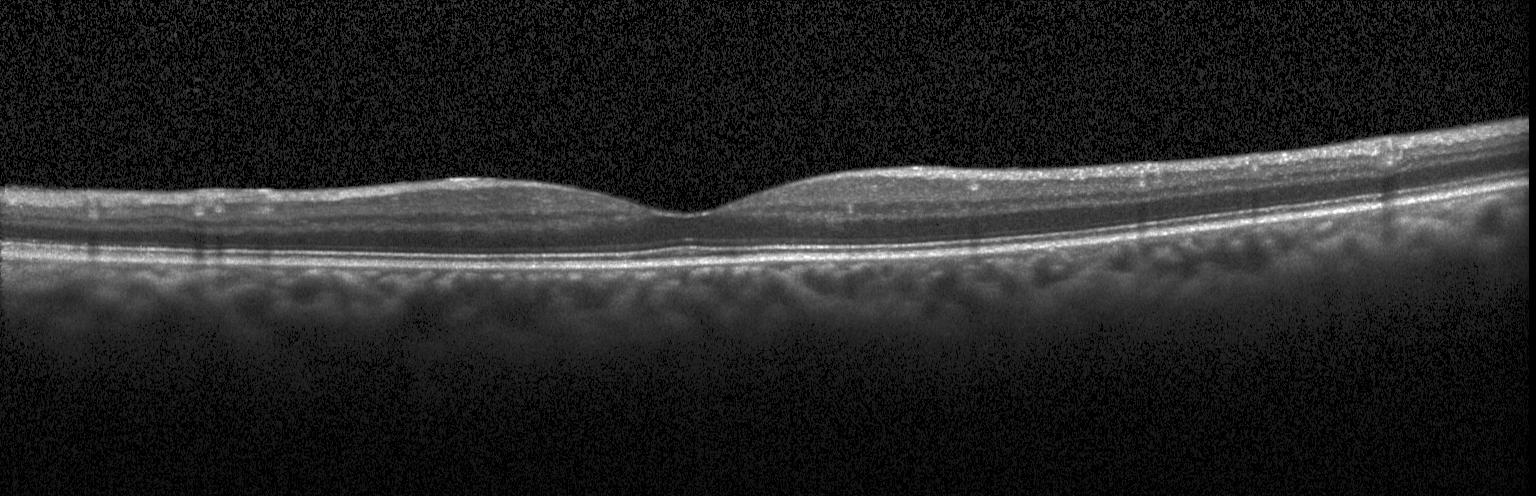
Diagnosis: no choroidal neovascularization, no diabetic macular edema, and no drusen.